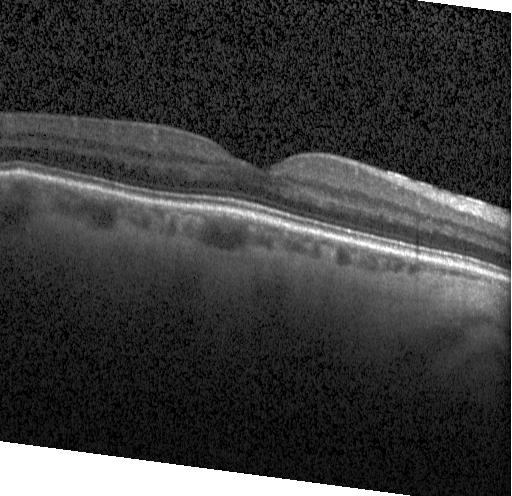

Fovea-centered · optical coherence tomography scan. Assessment: neither choroidal neovascularization, diabetic macular edema, nor drusen.